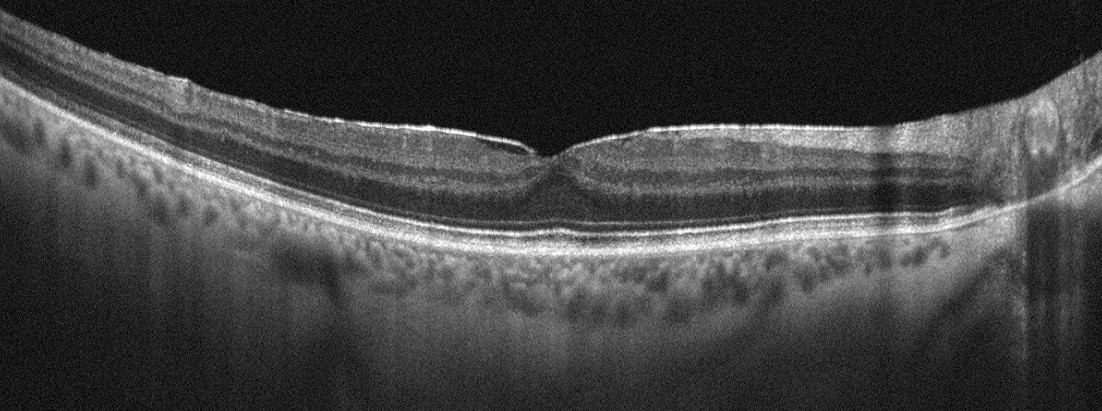

Instrument: Optovue Avanti RTVue XR, through the macula, retinal OCT B-scan.
Diagnosis: ERM.